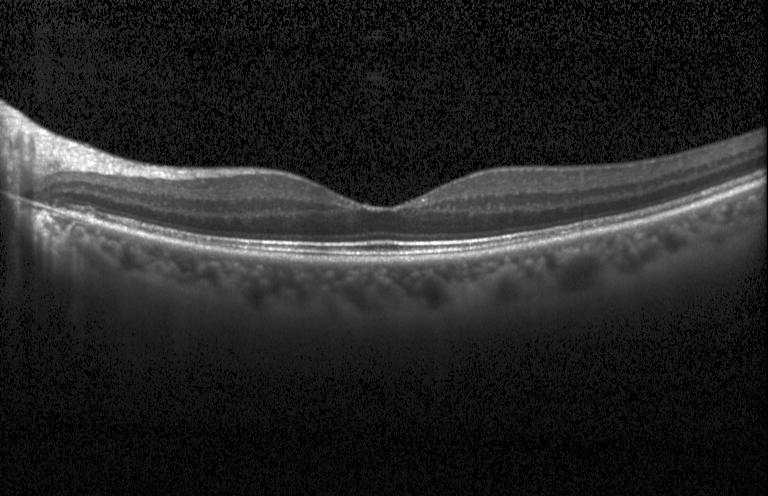
Through the macula; Heidelberg Spectralis; retinal OCT cross-section — Impression: no choroidal neovascularization, no diabetic macular edema, and no drusen.